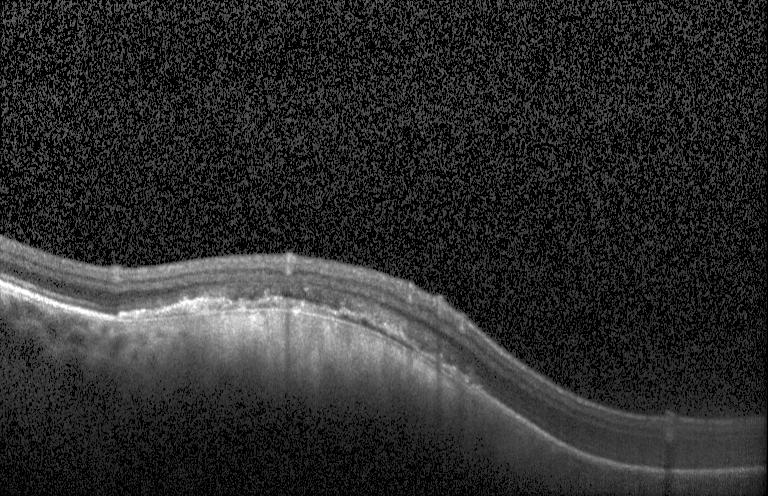

Macular OCT: choroidal neovascularization.